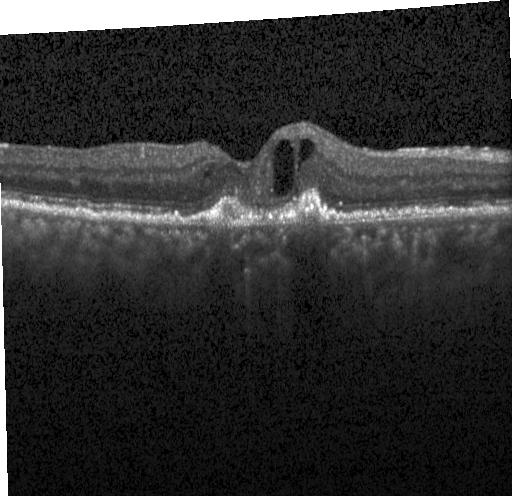
Spectral-domain optical coherence tomography; macular scan; optical coherence tomography scan.
Impression: a choroidal neovascular membrane.